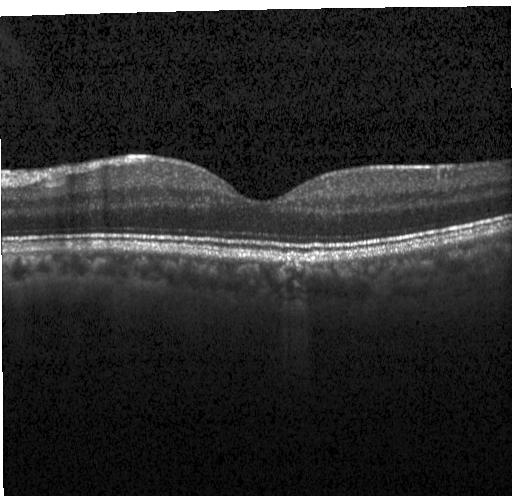 Macular OCT demonstrating no evidence of choroidal neovascularization, diabetic macular edema, or drusen.